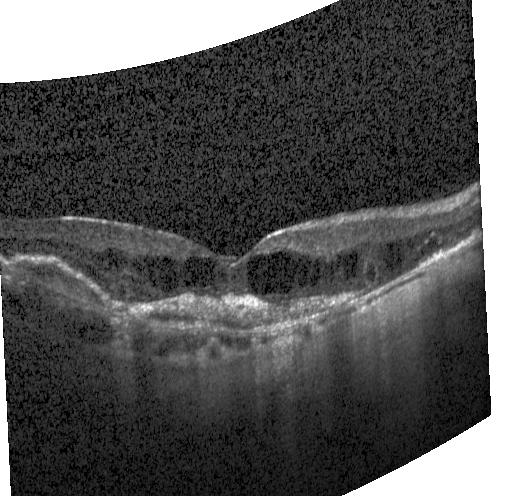
Spectral-domain optical coherence tomography, macular scan, OCT B-scan, instrument: Heidelberg Spectralis. A choroidal neovascular membrane.